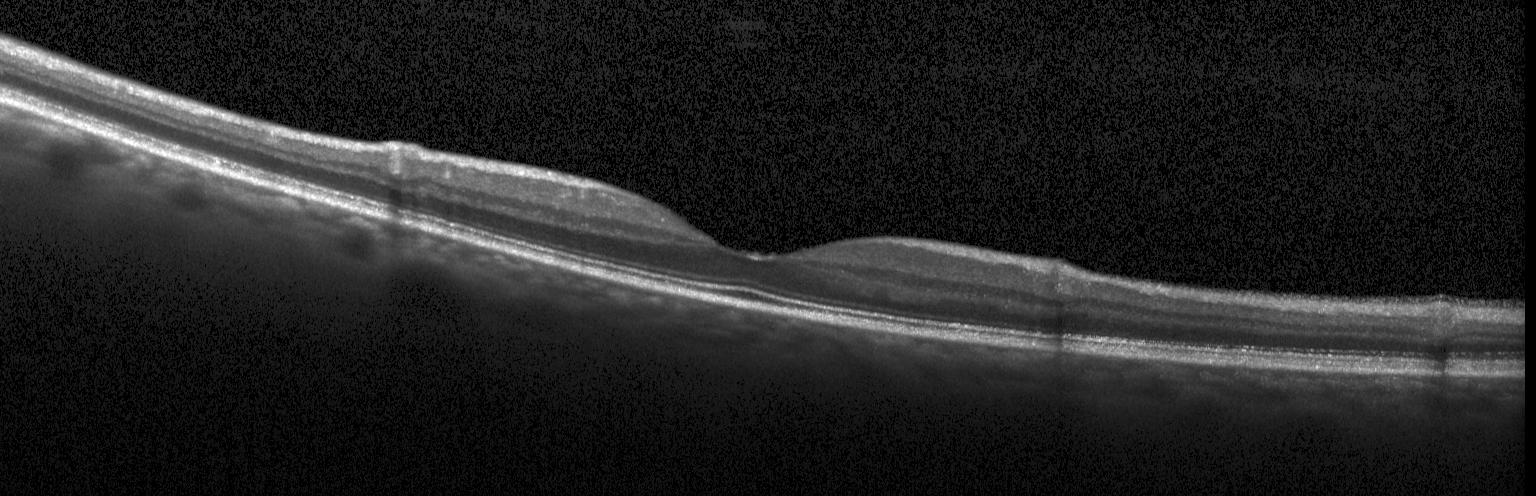 Heidelberg Spectralis OCT system. OCT B-scan. Through the macula. Finding: no choroidal neovascularization, no diabetic macular edema, and no drusen.